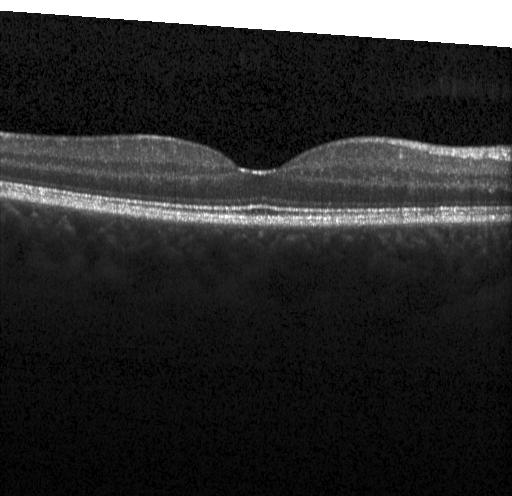

Acquired on a Heidelberg Spectralis; macular scan; retinal OCT cross-section; spectral-domain OCT. Diagnosis: no CNV, DME, or drusen.